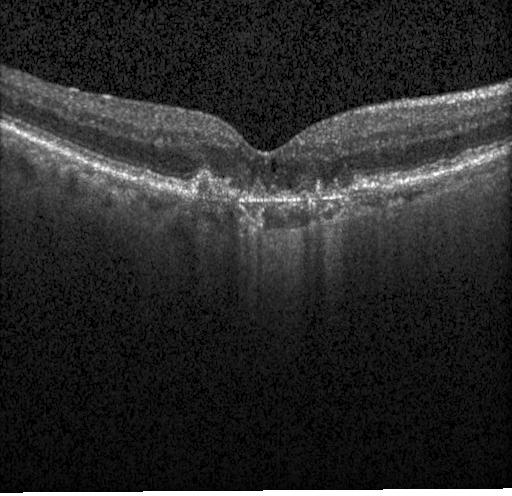

The scan shows a choroidal neovascular membrane.